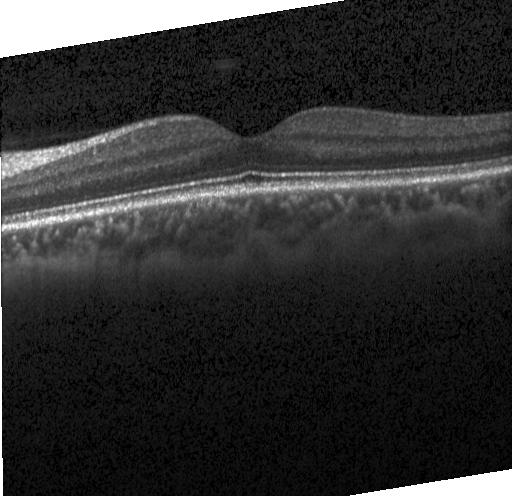

Impression: no evidence of choroidal neovascularization, diabetic macular edema, or drusen.